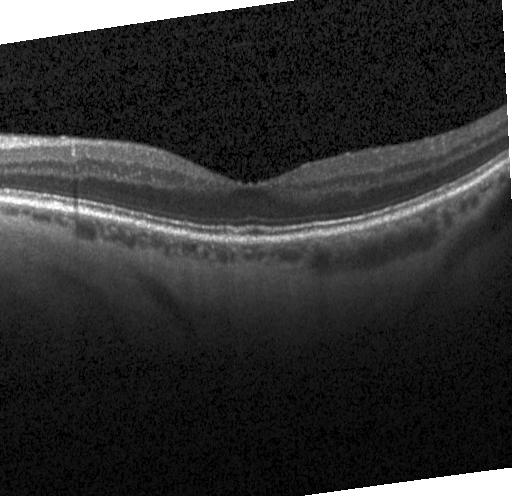 Fovea-centered; optical coherence tomography scan; SD-OCT; instrument: Heidelberg Spectralis
Diagnosis: no choroidal neovascularization, no diabetic macular edema, and no drusen.